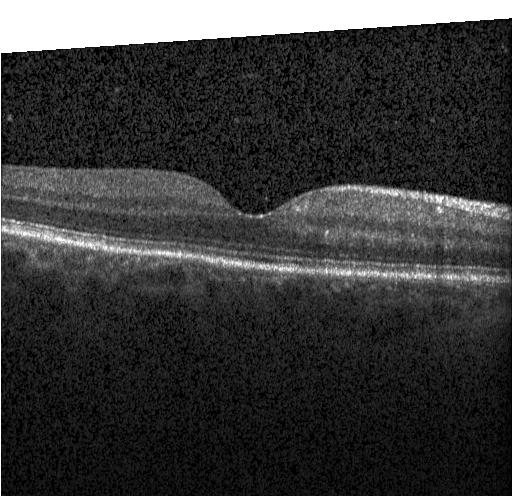

Assessment: neither CNV, DME, nor drusen.